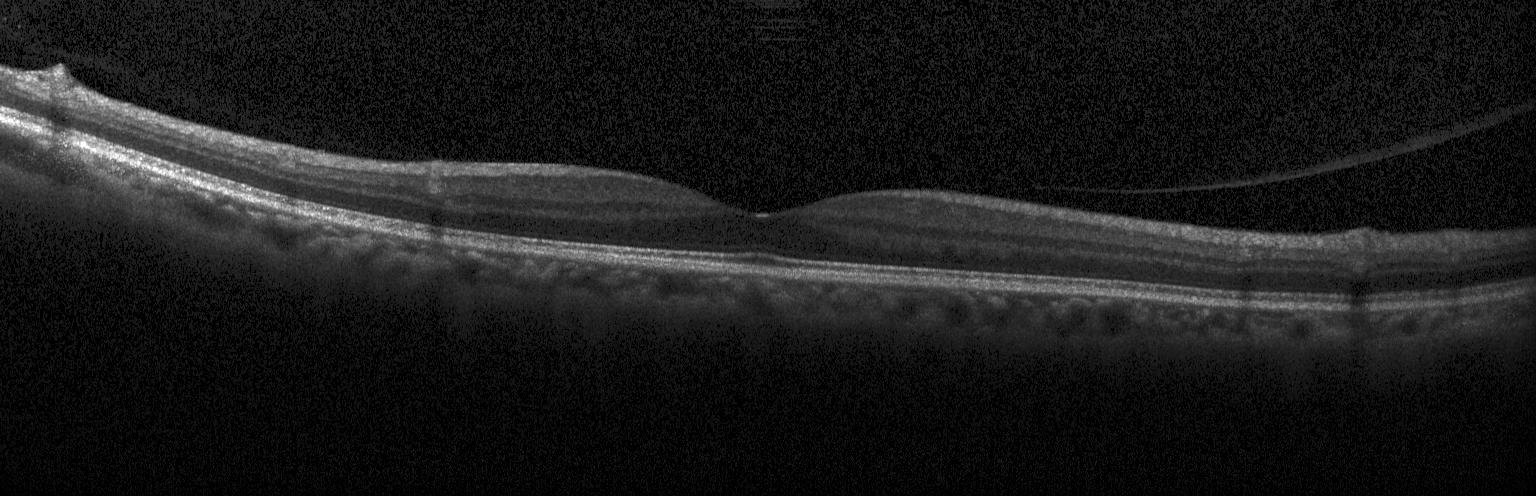 Diagnosis: no choroidal neovascularization, diabetic macular edema, or drusen.